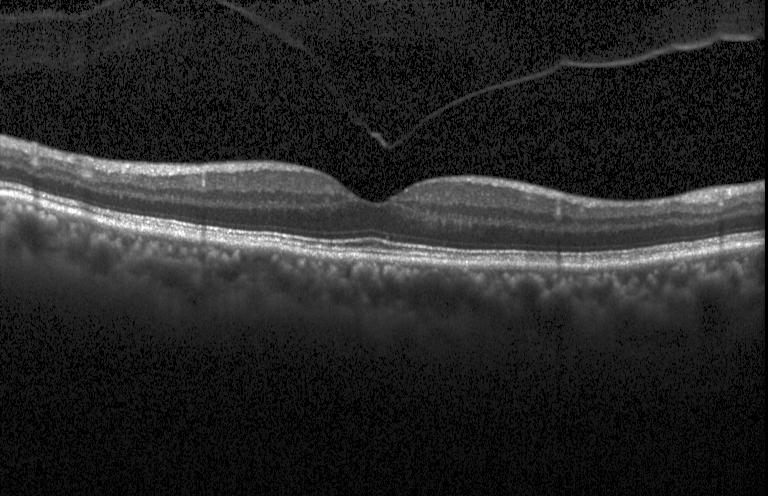

OCT finding: no choroidal neovascularization, no diabetic macular edema, and no drusen.